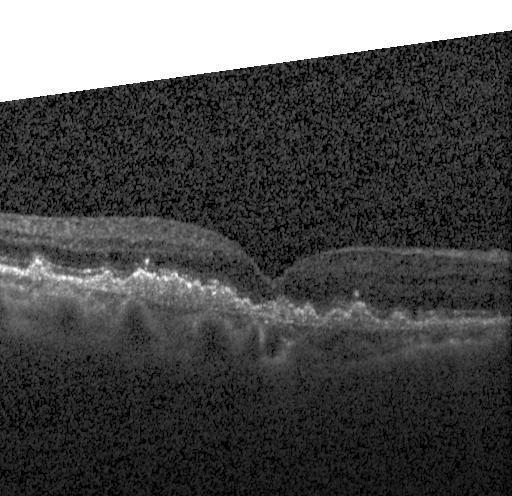
SD-OCT · retinal OCT B-scan · centered on the fovea · acquired on a Heidelberg Spectralis — Choroidal neovascularization.